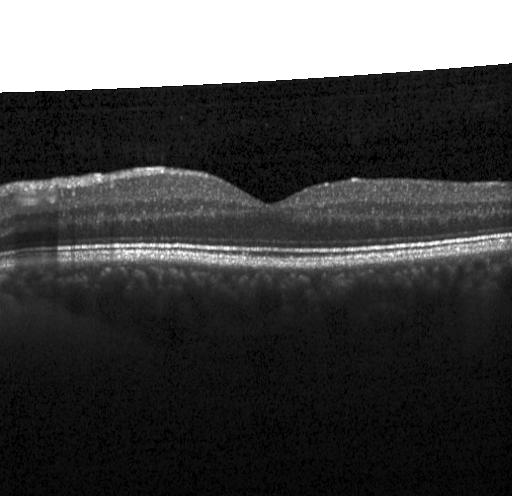 Impression: no choroidal neovascularization, no diabetic macular edema, and no drusen.